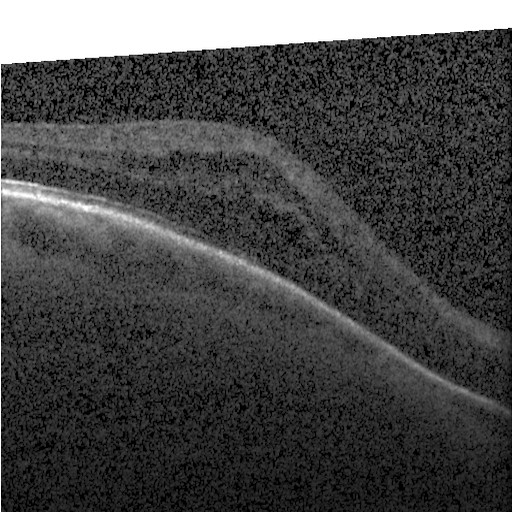 Retinal OCT B-scan · SD-OCT — Finding: diabetic macular edema (DME).